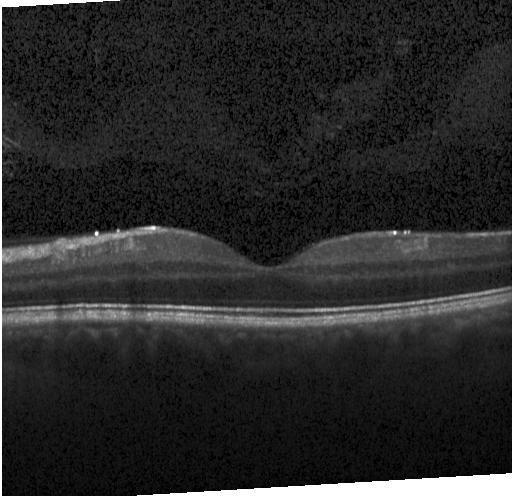
Spectral-domain OCT; OCT B-scan; fovea-centered
Finding: no CNV, no DME, and no drusen.